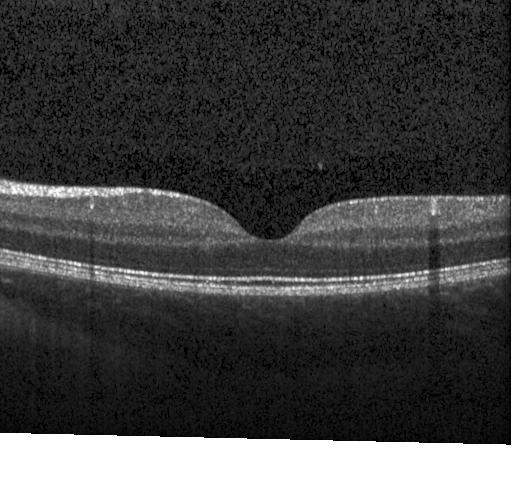 SD-OCT. Horizontal scan through the fovea. OCT line scan. Instrument: Heidelberg Spectralis.
Finding: no choroidal neovascularization, no diabetic macular edema, and no drusen.